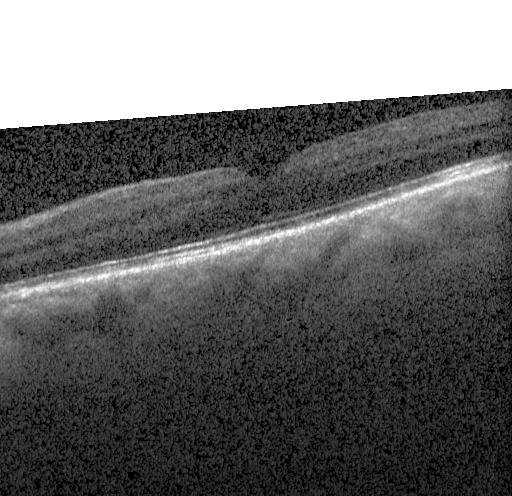 The scan shows neither CNV, DME, nor drusen.